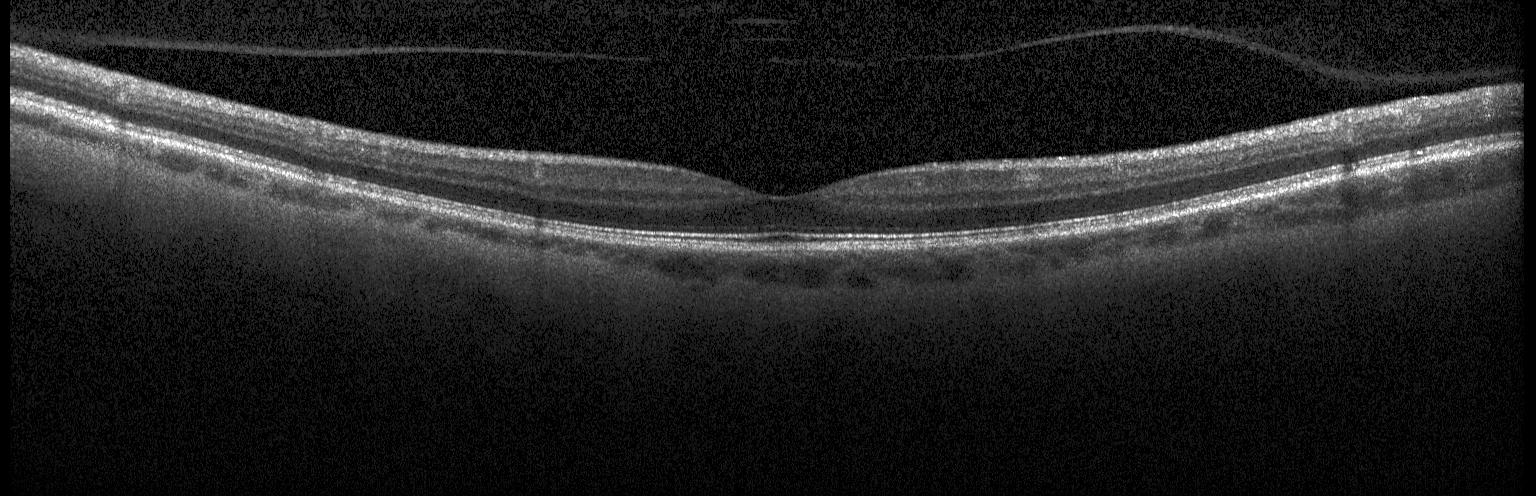 Retinal OCT B-scan · macular scan · instrument: Heidelberg Spectralis. No choroidal neovascularization, diabetic macular edema, or drusen.